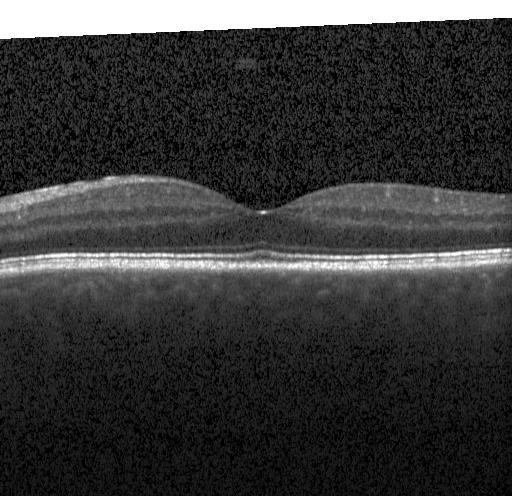 Impression: no CNV, DME, or drusen.